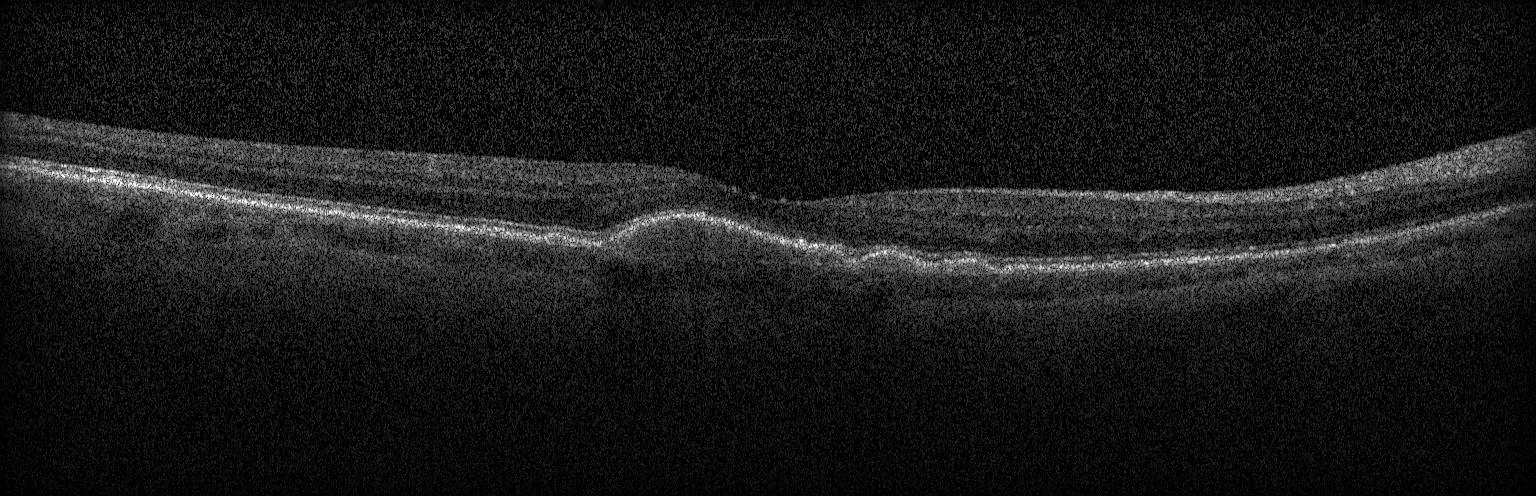

A choroidal neovascular membrane.